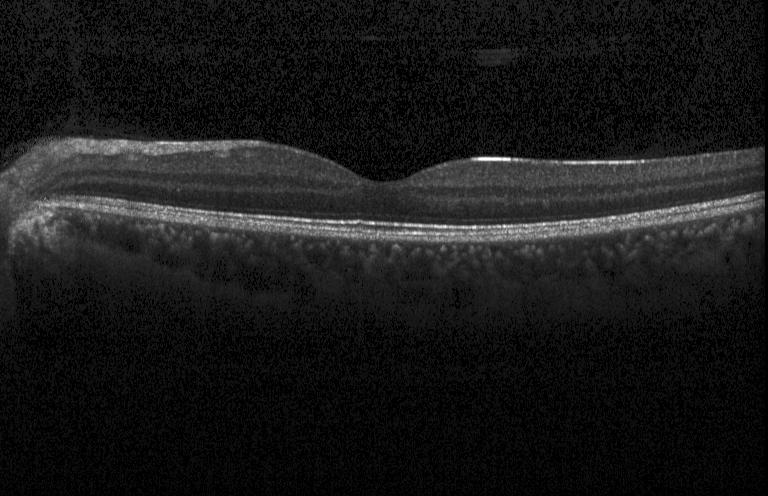

Heidelberg Spectralis. SD-OCT. Optical coherence tomography B-scan.
Macular OCT: no CNV, no DME, and no drusen.